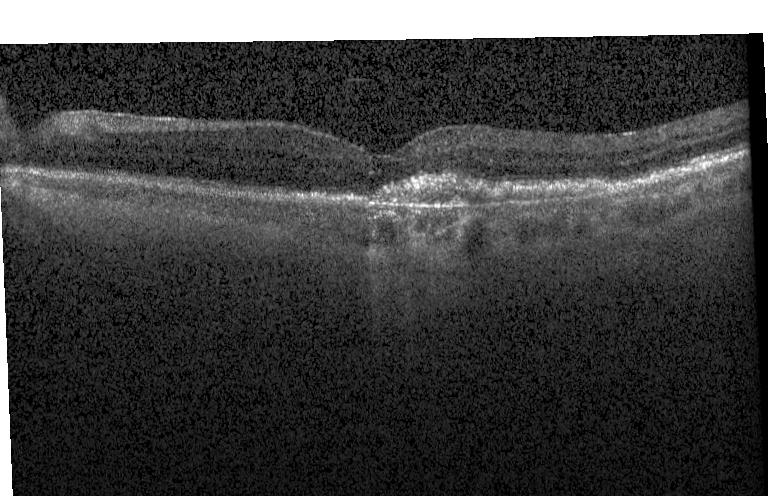
Impression: choroidal neovascularization.